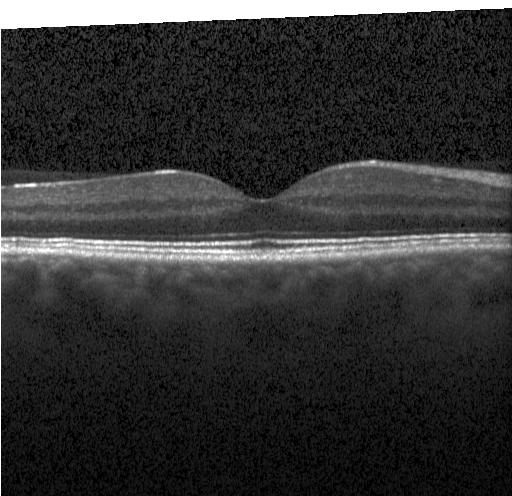
Retinal OCT B-scan — The scan shows no evidence of CNV, DME, or drusen.